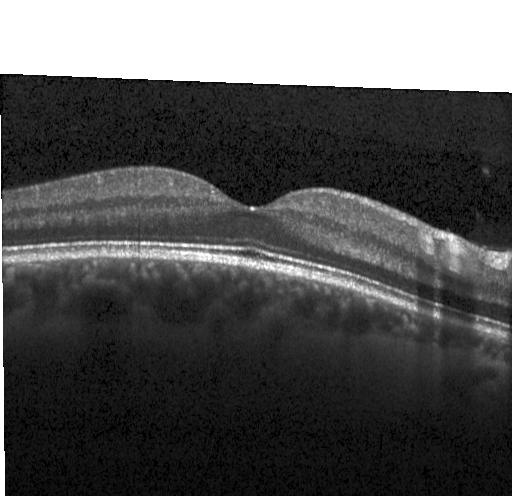

Heidelberg Spectralis · optical coherence tomography B-scan
Impression: no evidence of CNV, DME, or drusen.